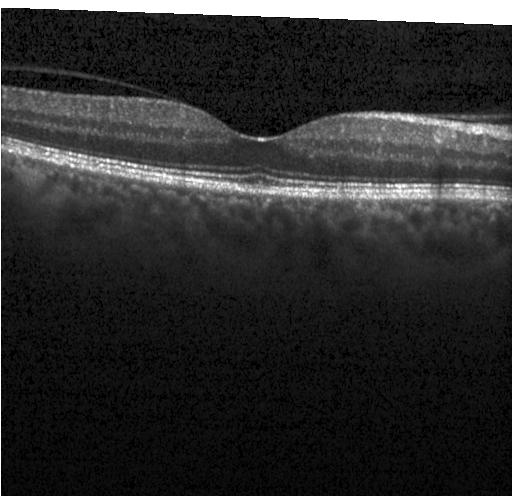
Optical coherence tomography B-scan.
OCT finding: no CNV, DME, or drusen.